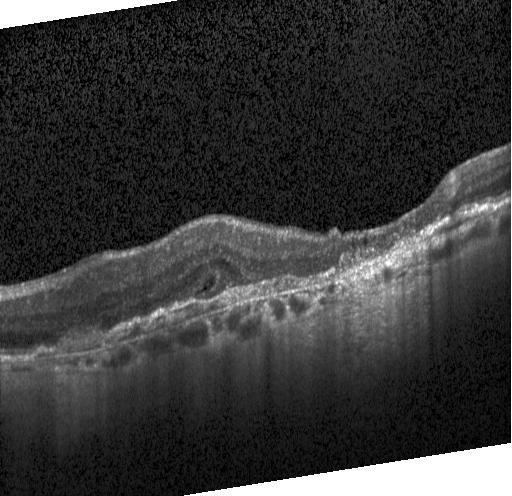

OCT scan showing CNV.